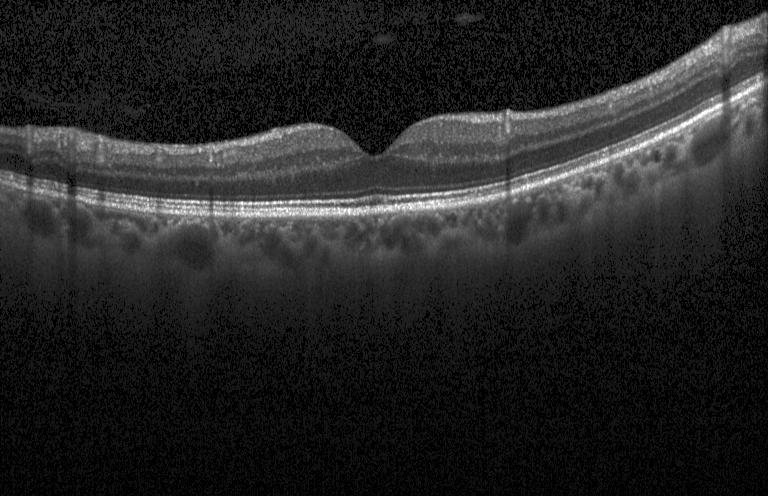 Spectral-domain OCT; optical coherence tomography B-scan
Macular OCT: neither choroidal neovascularization, diabetic macular edema, nor drusen.